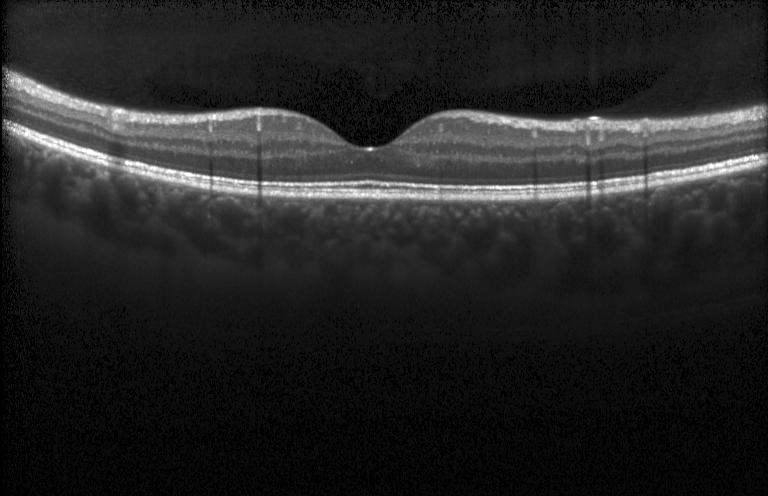

Optical coherence tomography scan. Spectral-domain OCT. Centered on the fovea. Acquired on a Heidelberg Spectralis.
Macular OCT: no choroidal neovascularization, no diabetic macular edema, and no drusen.